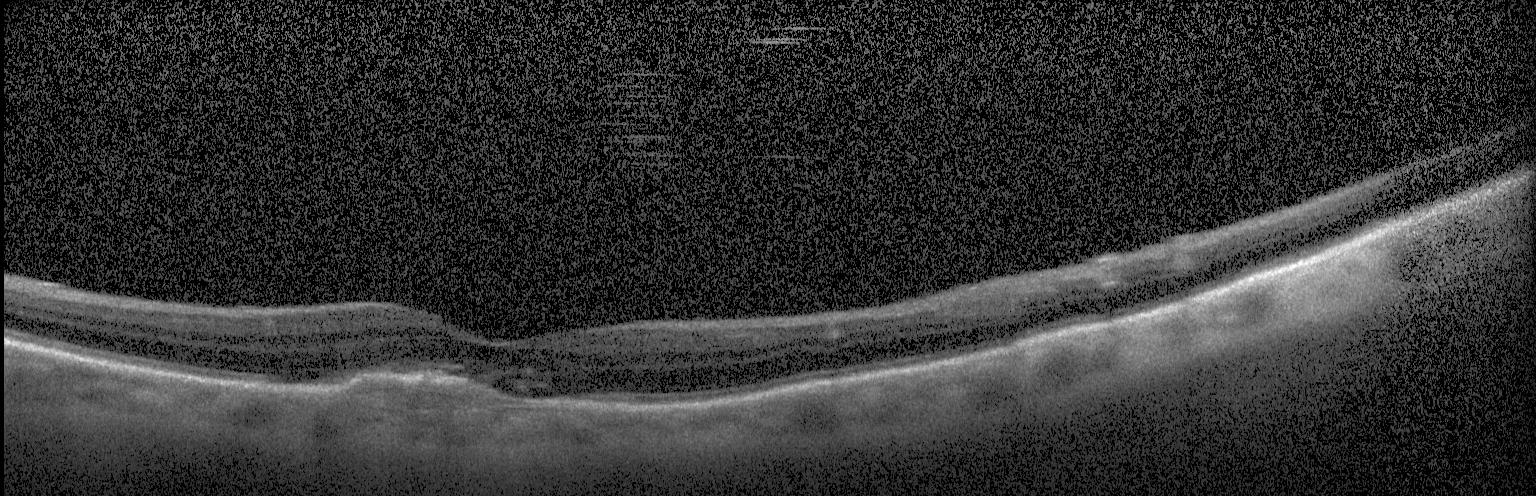 Acquired on a Heidelberg Spectralis, optical coherence tomography B-scan, spectral-domain OCT, centered on the fovea — This B-scan demonstrates a choroidal neovascular membrane.